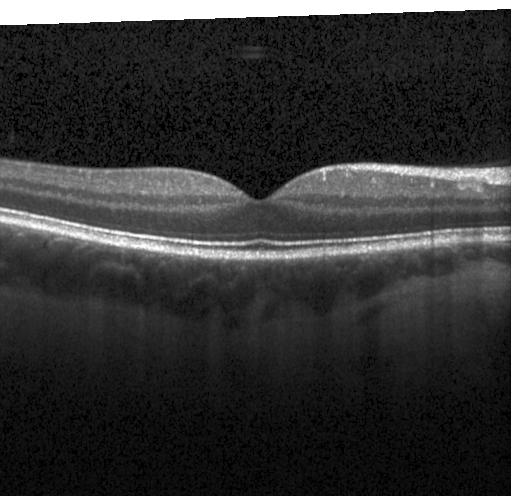

Macular OCT: no choroidal neovascularization, no diabetic macular edema, and no drusen.